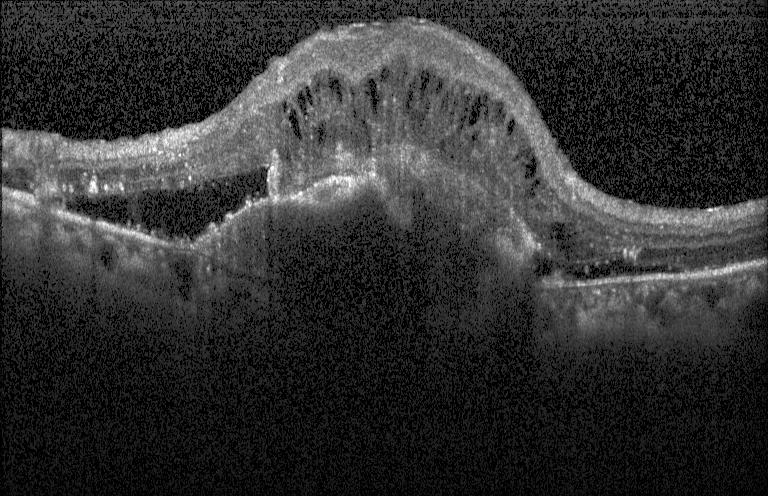

Retinal OCT cross-section. Heidelberg Spectralis OCT system.
Impression: choroidal neovascularization.